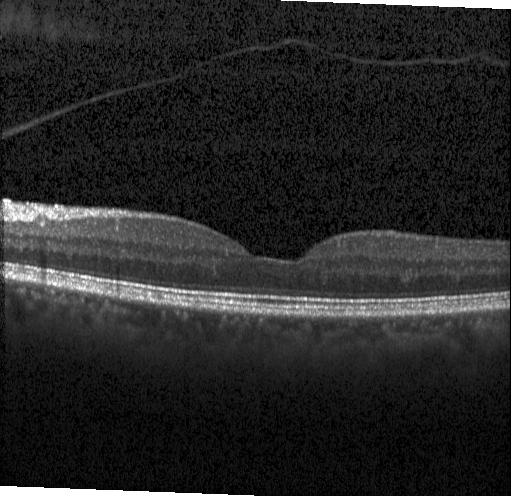
Finding: neither choroidal neovascularization, diabetic macular edema, nor drusen.